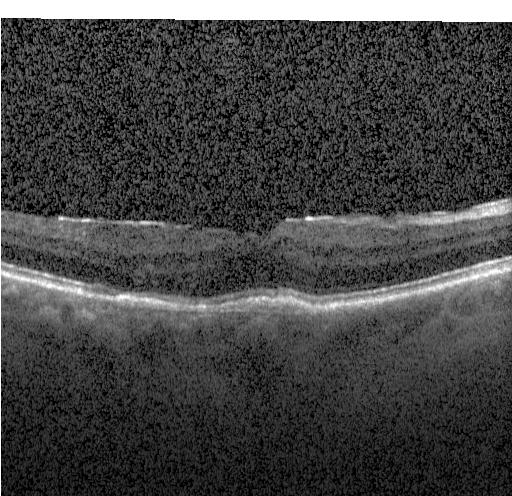
Diagnosis: a choroidal neovascular membrane.